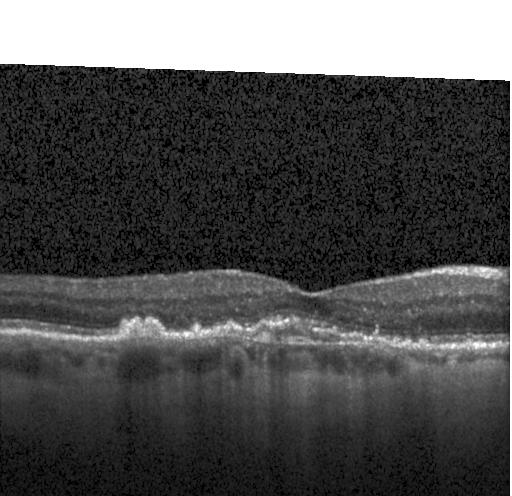
Acquired on a Heidelberg Spectralis; retinal OCT cross-section; spectral-domain OCT — Impression: choroidal neovascularization (CNV).